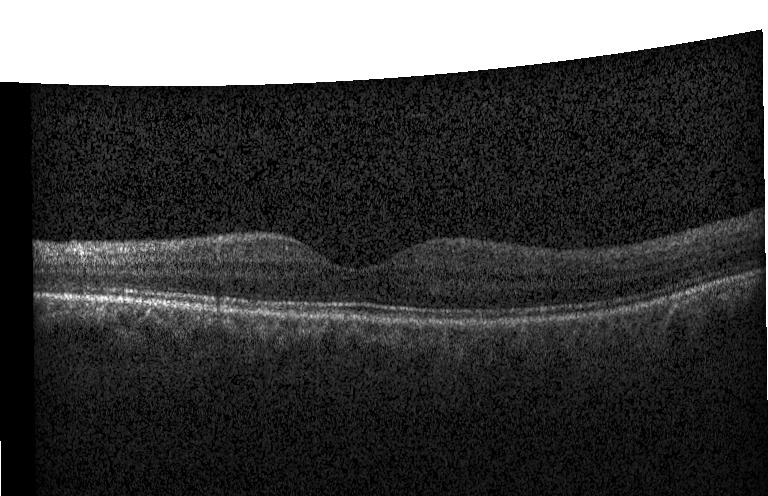 Centered on the fovea · OCT line scan.
Diagnosis: neither CNV, DME, nor drusen.